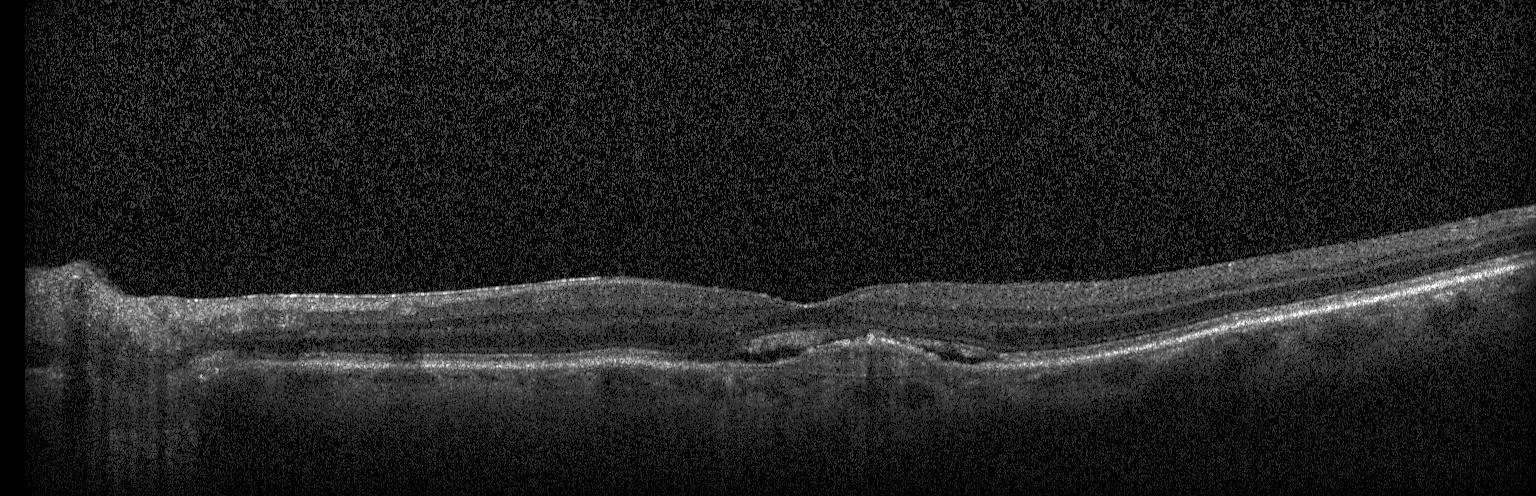
OCT B-scan — Macular OCT: a choroidal neovascular membrane.